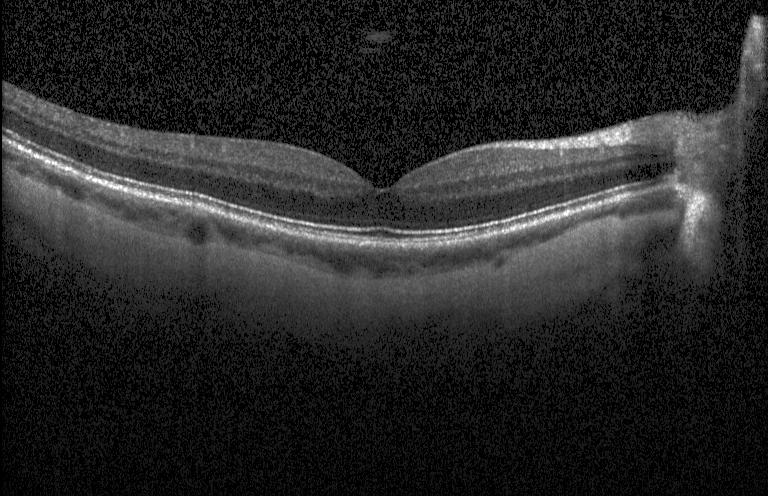 Spectral-domain OCT; optical coherence tomography scan; instrument: Heidelberg Spectralis — Diagnosis: no evidence of choroidal neovascularization, diabetic macular edema, or drusen.